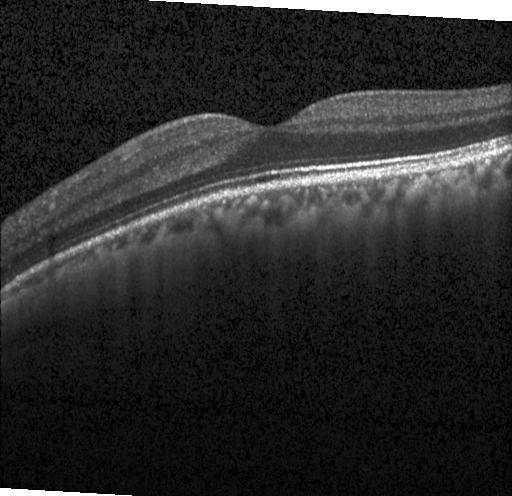

Retinal OCT cross-section showing neither CNV, DME, nor drusen.